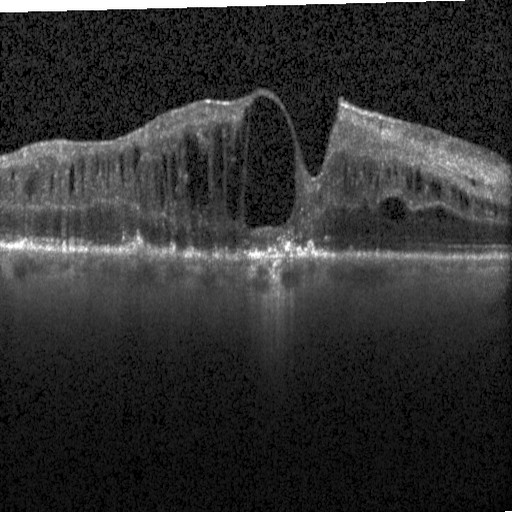 Heidelberg Spectralis, retinal OCT B-scan, spectral-domain optical coherence tomography.
Finding: DME.